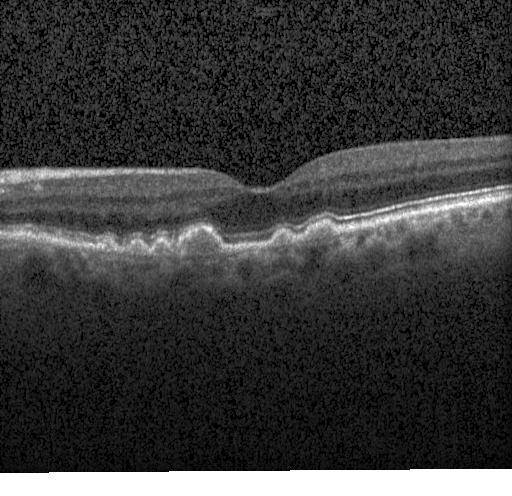

Spectral-domain optical coherence tomography; centered on the fovea; Heidelberg Spectralis OCT system; optical coherence tomography scan — Assessment: multiple drusen.